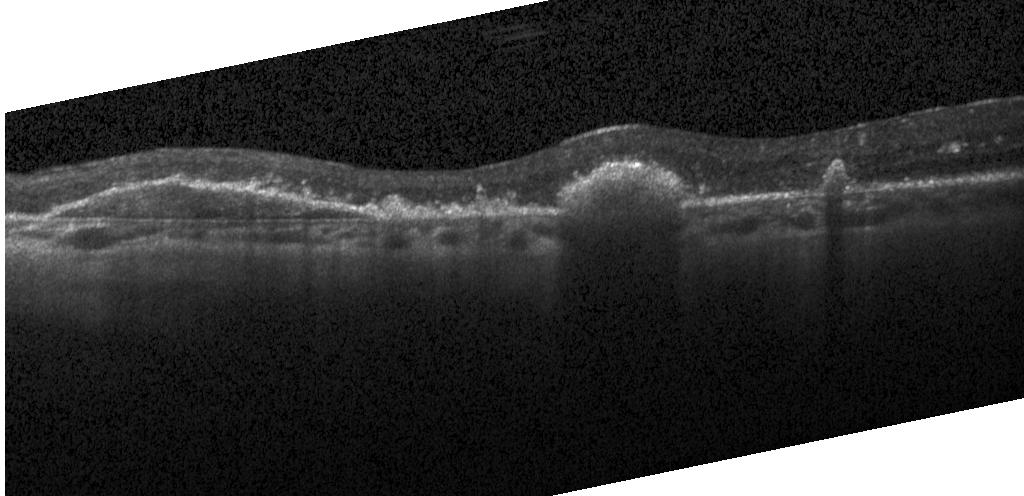

Heidelberg Spectralis; fovea-centered; optical coherence tomography B-scan; spectral-domain OCT.
The scan shows choroidal neovascularization (CNV).